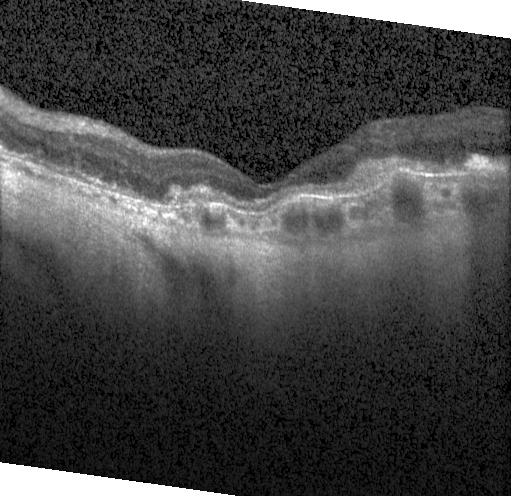 Through the macula; OCT B-scan. Impression: a choroidal neovascular membrane.